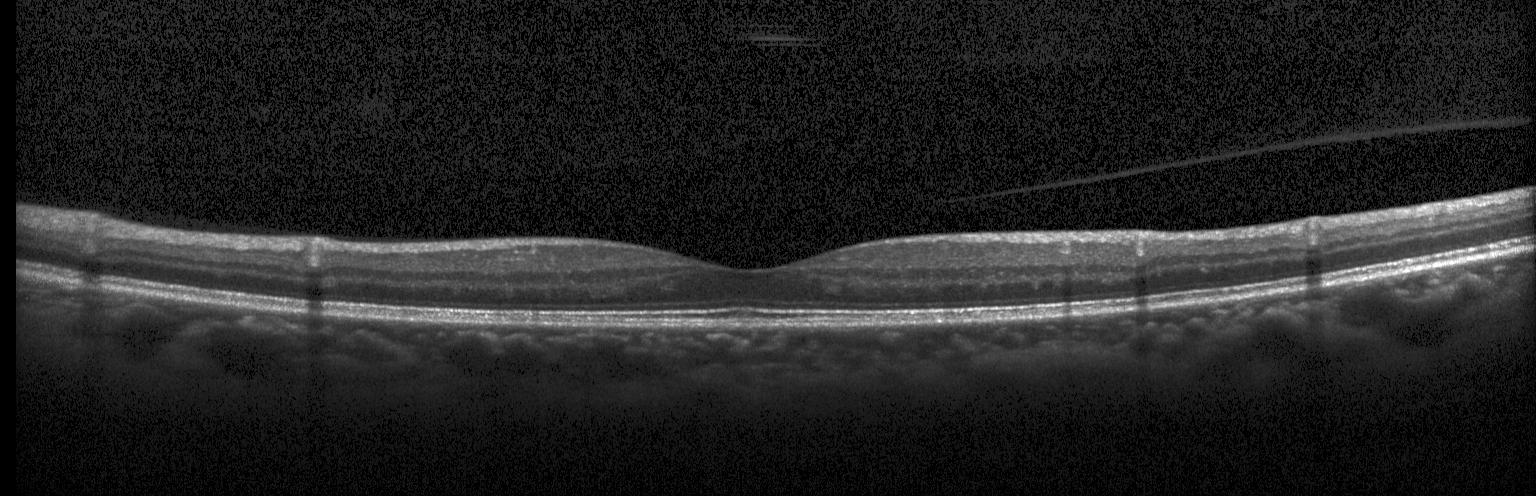

OCT finding: no choroidal neovascularization, no diabetic macular edema, and no drusen.